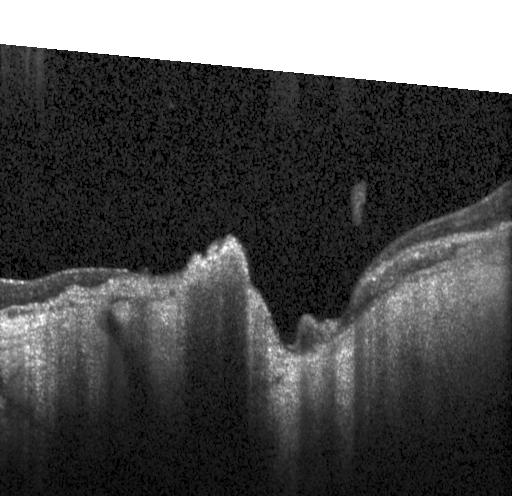
Optical coherence tomography scan; Heidelberg Spectralis; through the macula — Diagnosis: choroidal neovascularization (CNV).